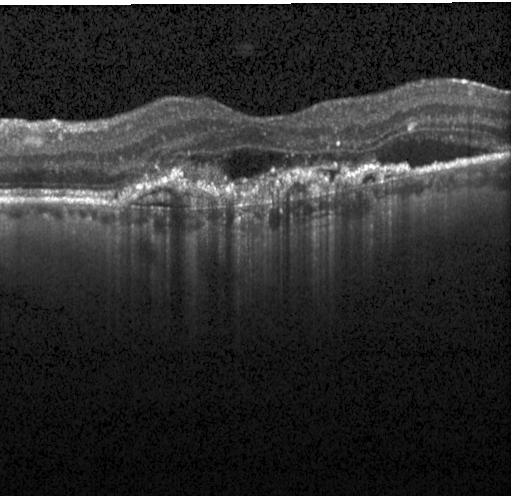 Centered on the fovea · spectral-domain OCT · OCT B-scan
Impression: choroidal neovascularization (CNV).